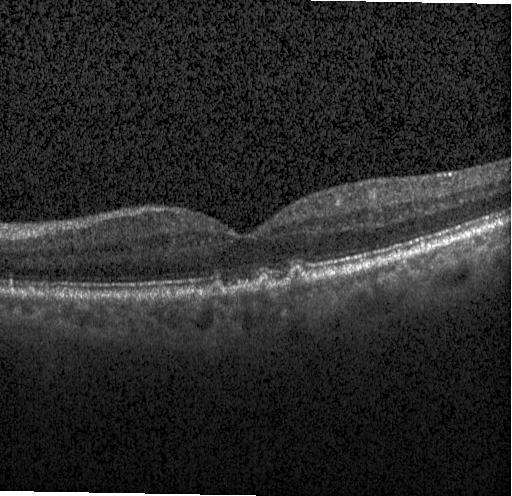
This B-scan demonstrates drusen.